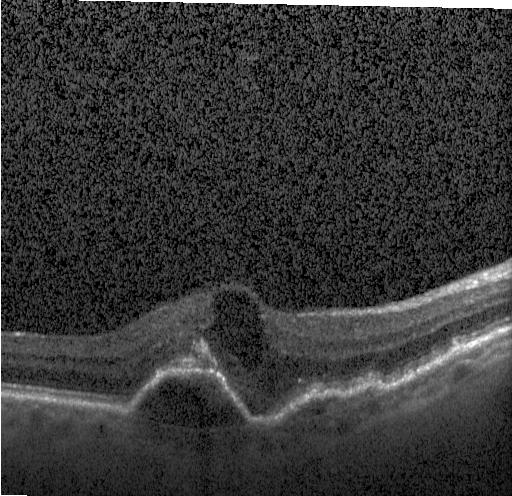
OCT B-scan
This B-scan demonstrates choroidal neovascularization.